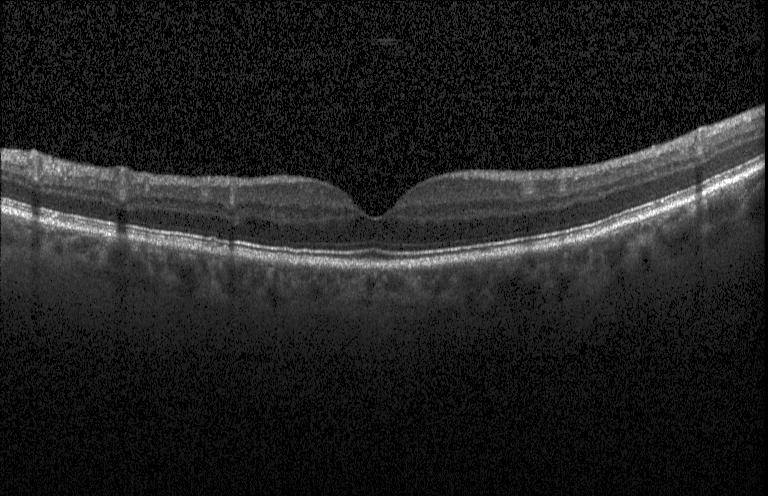

Retinal OCT B-scan. Through the macula. Instrument: Heidelberg Spectralis.
Diagnosis: neither choroidal neovascularization, diabetic macular edema, nor drusen.